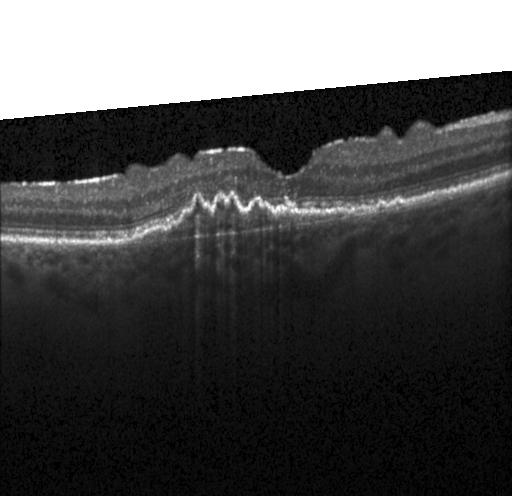 OCT B-scan. SD-OCT. The scan shows a choroidal neovascular membrane.